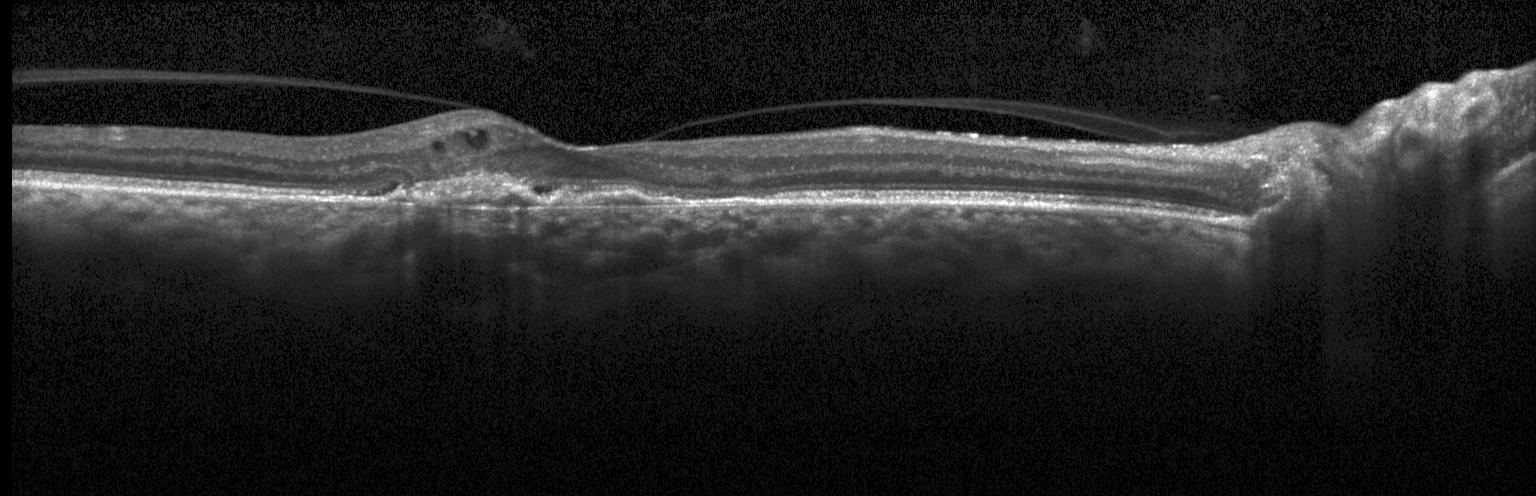
Retinal OCT B-scan.
Macular OCT: a choroidal neovascular membrane.